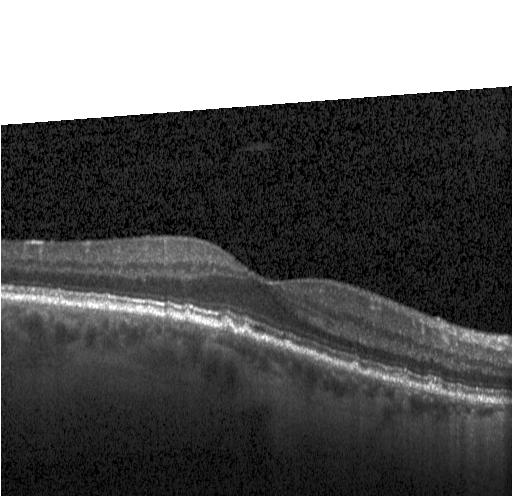 OCT scan showing multiple drusen.